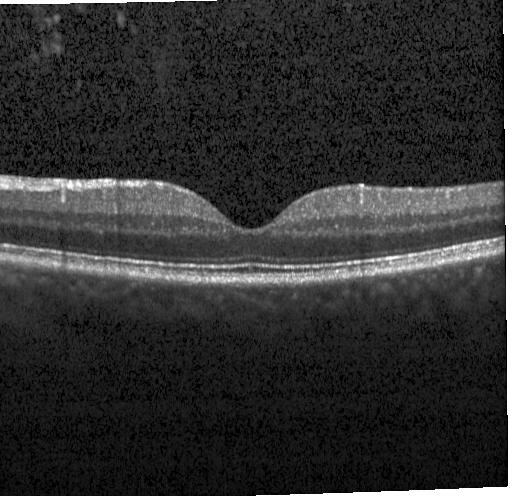
This B-scan demonstrates neither CNV, DME, nor drusen.